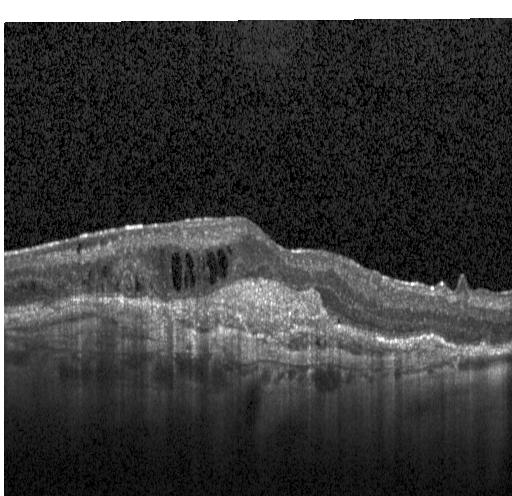

Optical coherence tomography scan; Heidelberg Spectralis; spectral-domain optical coherence tomography — CNV.